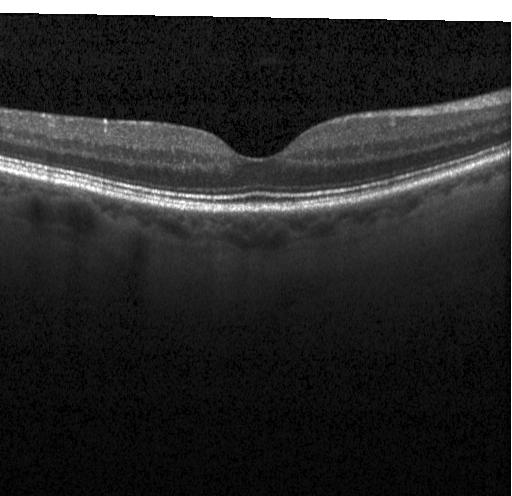

Optical coherence tomography B-scan
OCT finding: no CNV, no DME, and no drusen.